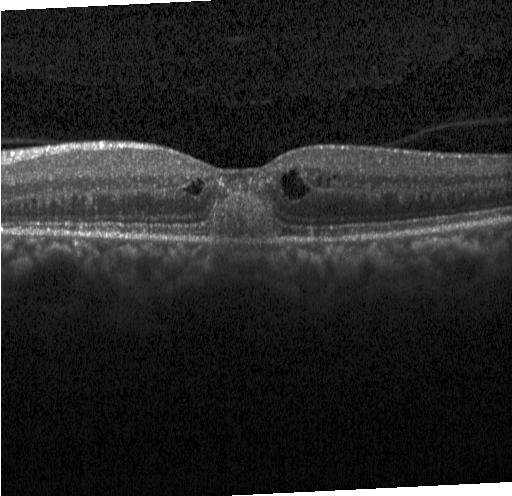
Spectral-domain optical coherence tomography; fovea-centered; optical coherence tomography B-scan — Assessment: CNV.